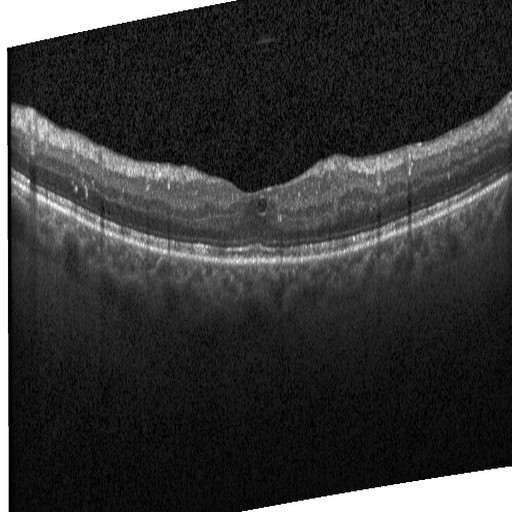
Spectral-domain OCT B-scan: diabetic macular edema (DME).